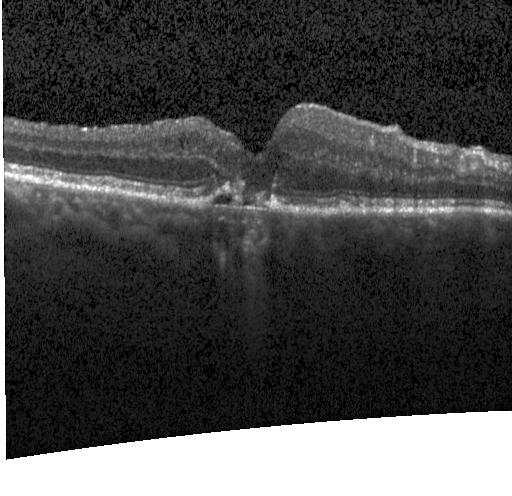

Heidelberg Spectralis OCT system. Spectral-domain optical coherence tomography. Through the macula. OCT B-scan. This B-scan demonstrates a choroidal neovascular membrane.